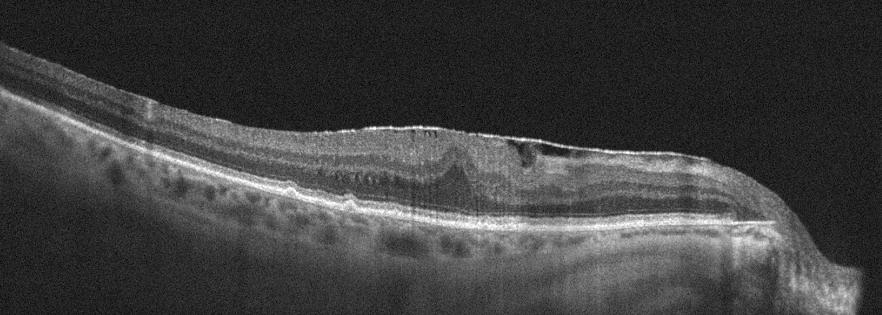 Retinal OCT B-scan, right eye.
OCT finding: ERM.